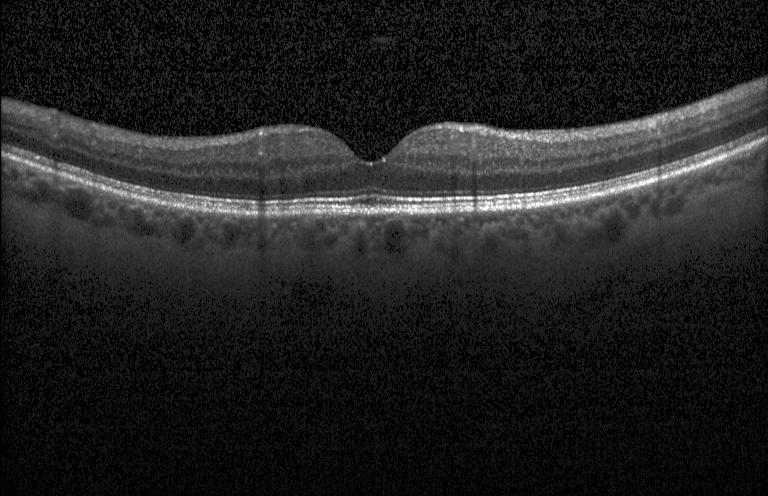
Optical coherence tomography scan. Finding: no choroidal neovascularization, no diabetic macular edema, and no drusen.